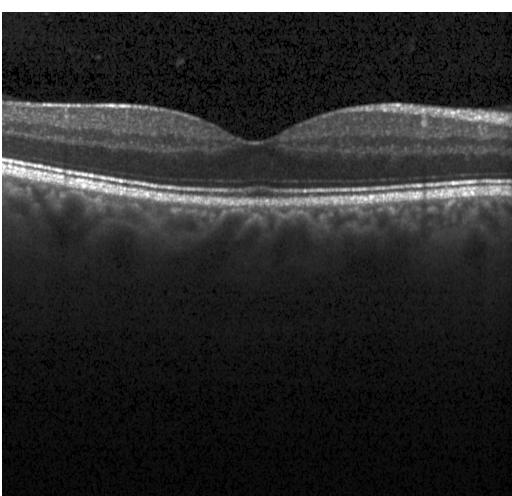
Macular OCT demonstrating neither choroidal neovascularization, diabetic macular edema, nor drusen.